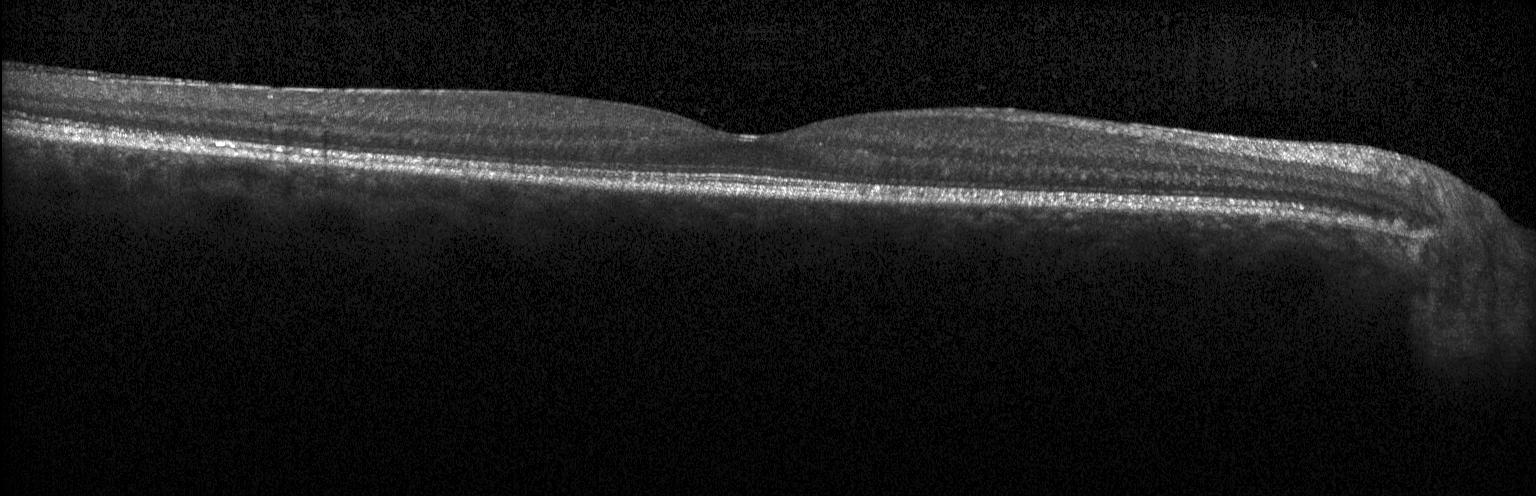 Retinal OCT B-scan. Neither CNV, DME, nor drusen.